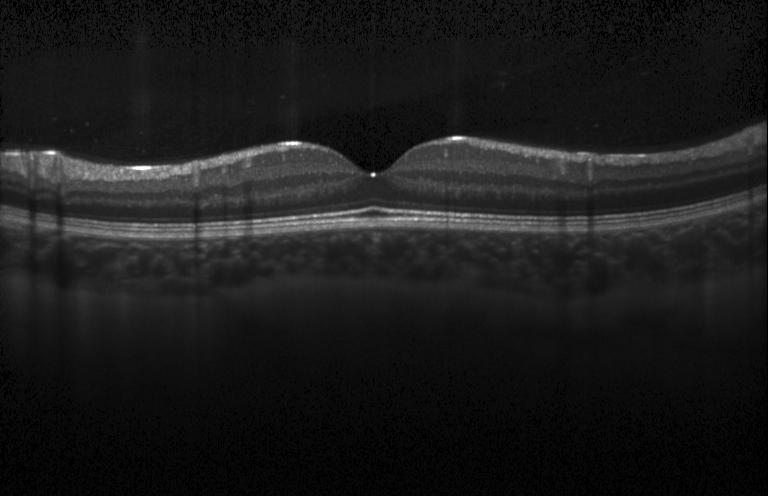

Optical coherence tomography B-scan, fovea-centered. Impression: no evidence of CNV, DME, or drusen.